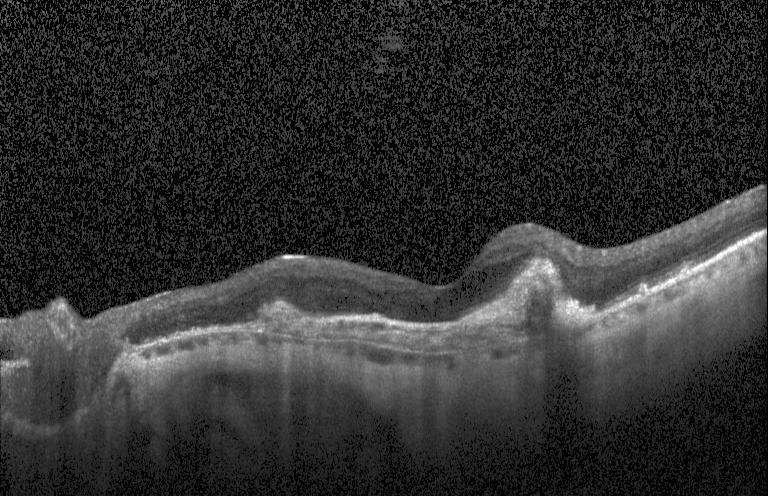
Spectral-domain OCT B-scan: CNV.